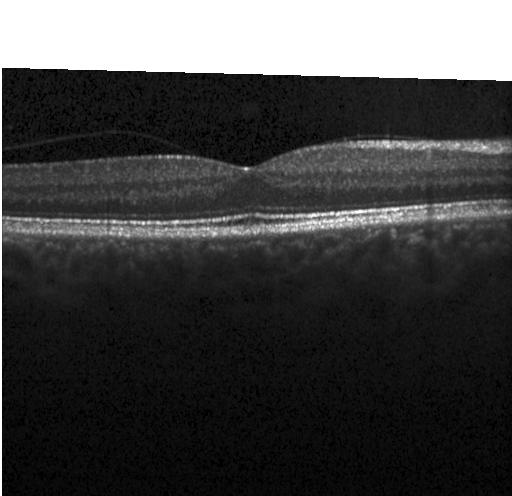 Instrument: Heidelberg Spectralis; optical coherence tomography scan; centered on the fovea; SD-OCT
Assessment: no evidence of CNV, DME, or drusen.